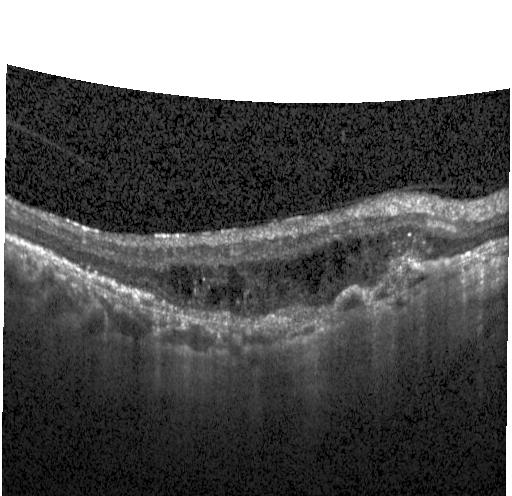
Spectral-domain optical coherence tomography · macular scan · optical coherence tomography B-scan · Heidelberg Spectralis OCT system — Finding: a choroidal neovascular membrane.